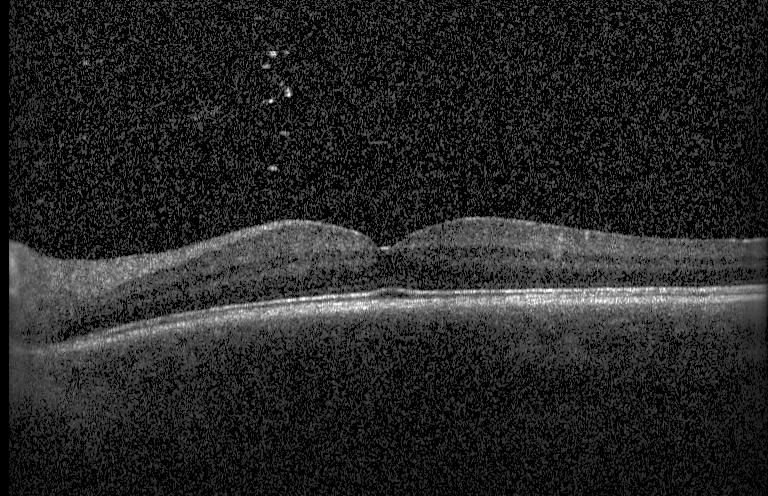

Spectral-domain optical coherence tomography · optical coherence tomography scan
Finding: no choroidal neovascularization, diabetic macular edema, or drusen.